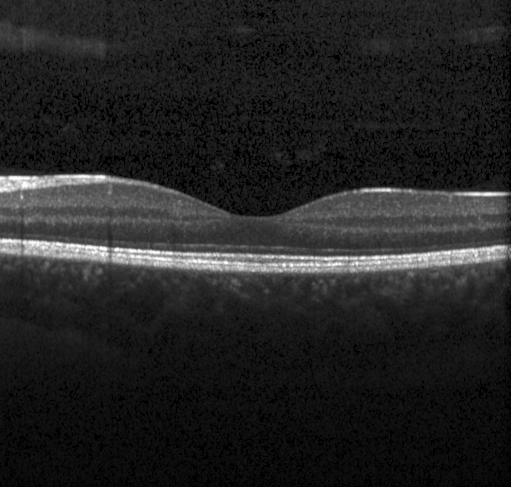

This B-scan demonstrates no evidence of choroidal neovascularization, diabetic macular edema, or drusen.